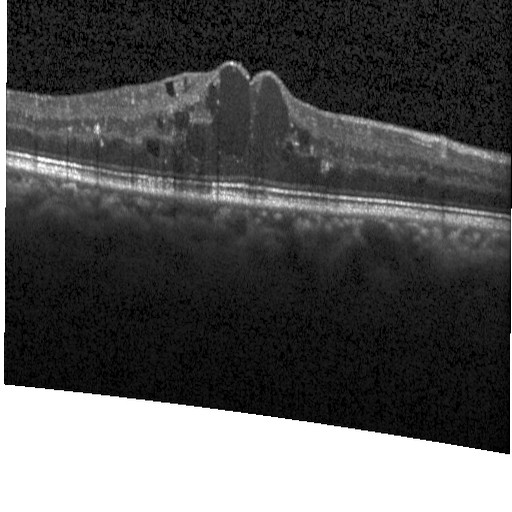 Spectral-domain OCT, fovea-centered, Heidelberg Spectralis OCT system, OCT line scan
Dx: DME.